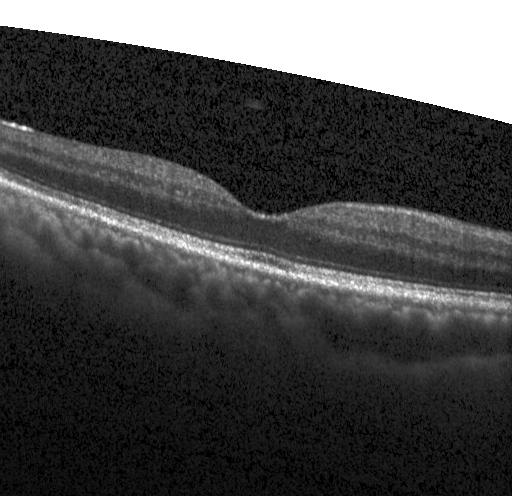
Impression: no choroidal neovascularization, no diabetic macular edema, and no drusen.